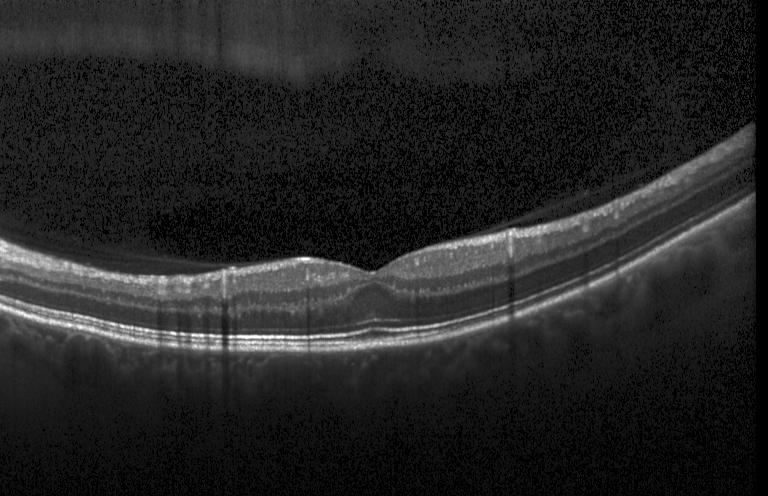

This B-scan demonstrates no choroidal neovascularization, diabetic macular edema, or drusen.